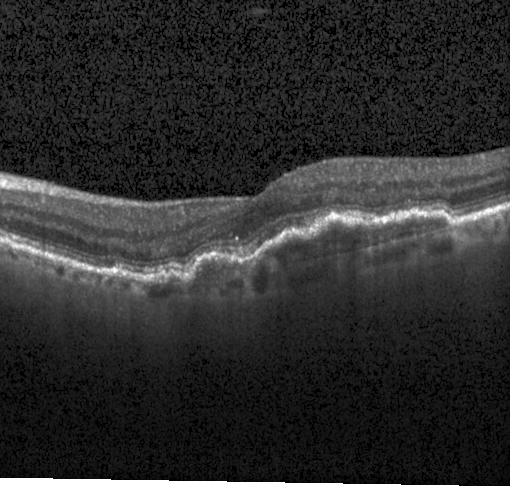
This B-scan demonstrates a choroidal neovascular membrane.